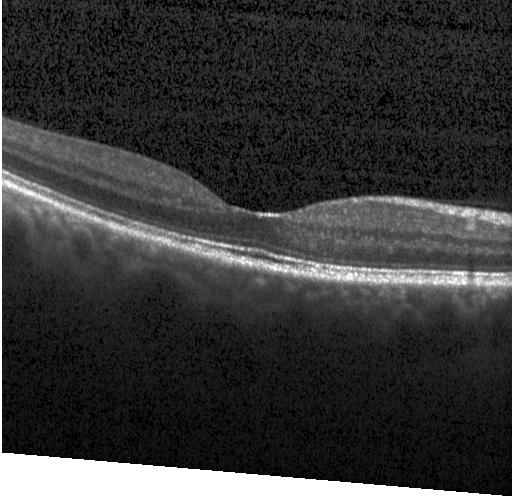 Optical coherence tomography scan; macular scan; instrument: Heidelberg Spectralis; SD-OCT
This B-scan demonstrates neither CNV, DME, nor drusen.